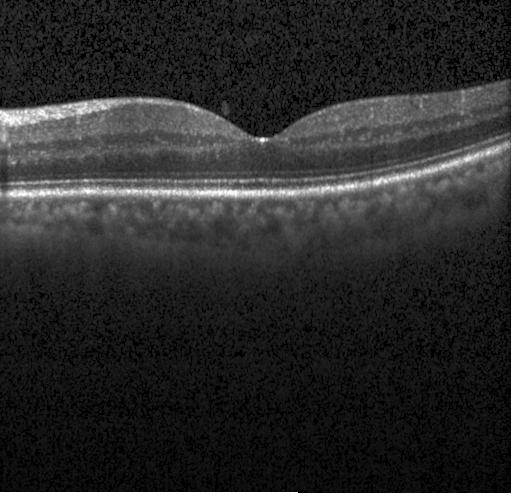

OCT B-scan
This B-scan demonstrates neither choroidal neovascularization, diabetic macular edema, nor drusen.